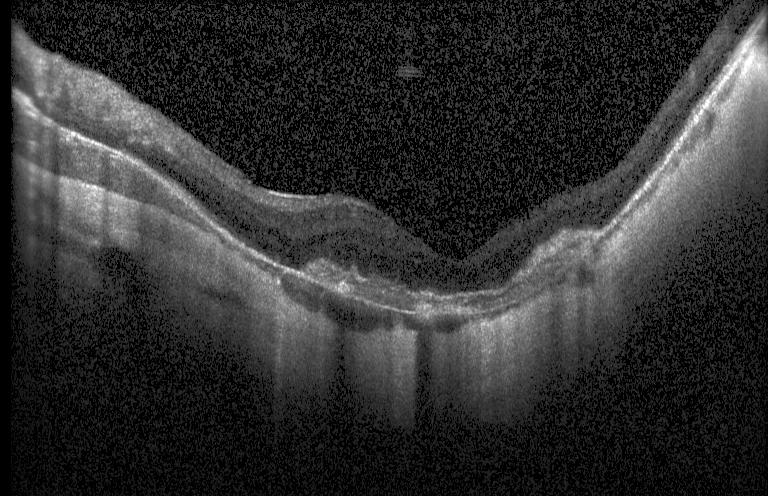 Diagnosis: CNV.